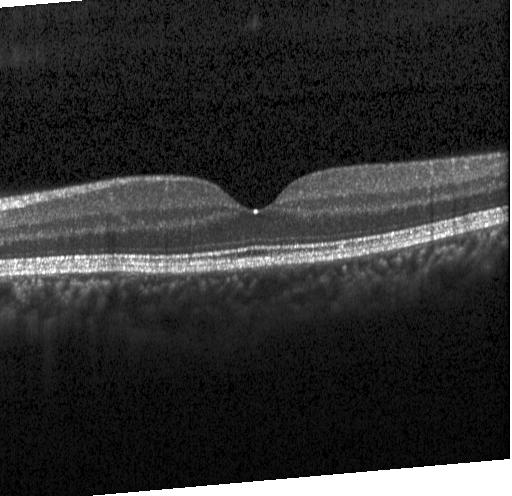 Finding: no CNV, no DME, and no drusen.